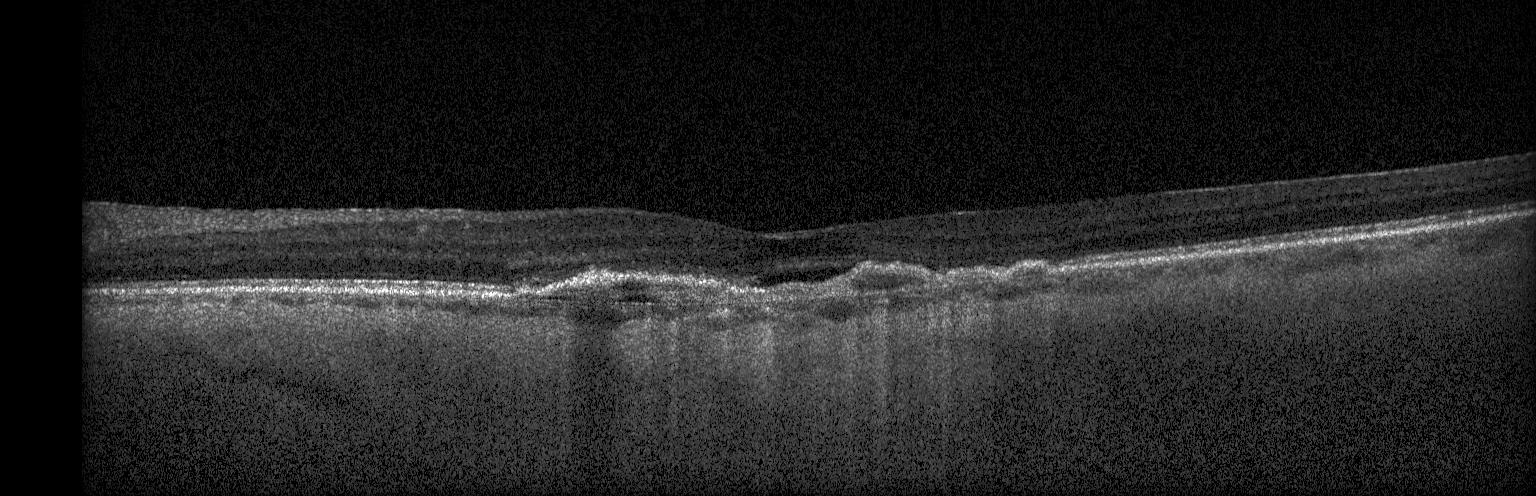

Acquired on a Heidelberg Spectralis. Optical coherence tomography scan. Fovea-centered. Spectral-domain OCT
Impression: a choroidal neovascular membrane.